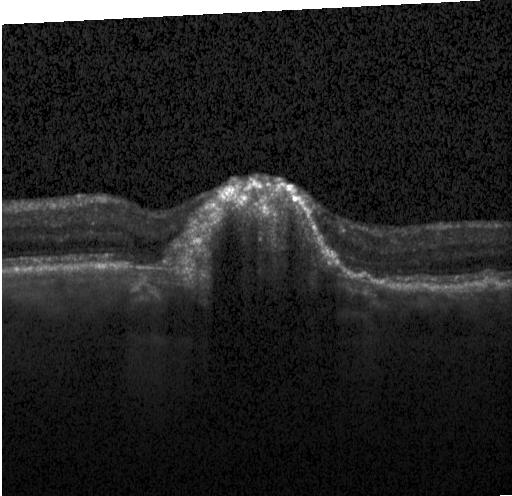
Acquired on a Heidelberg Spectralis · optical coherence tomography B-scan
A choroidal neovascular membrane.